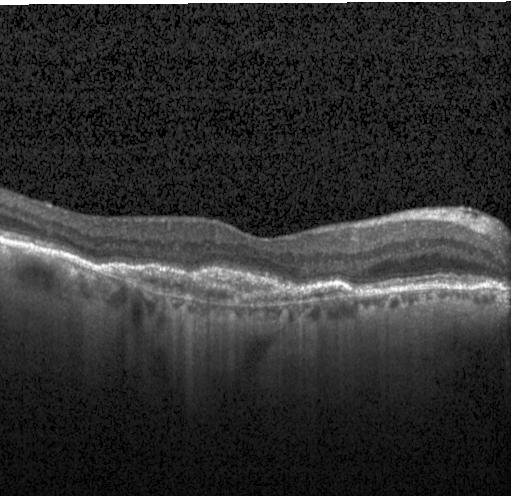

Optical coherence tomography B-scan.
Dx: a choroidal neovascular membrane.